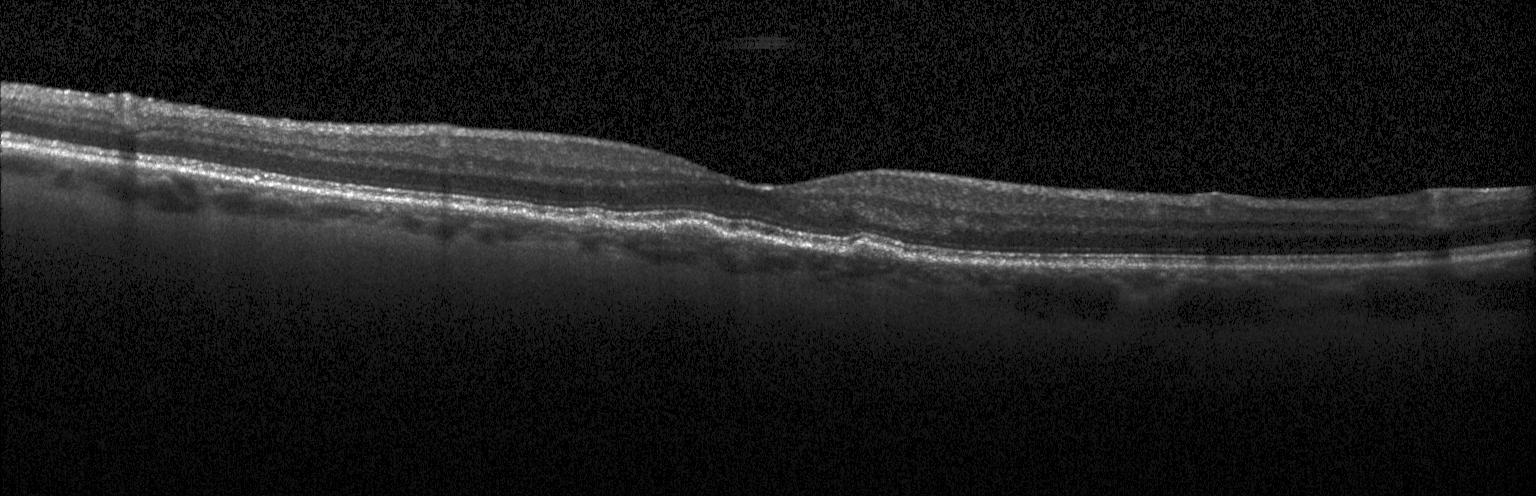

Finding: sub-RPE drusenoid deposits.